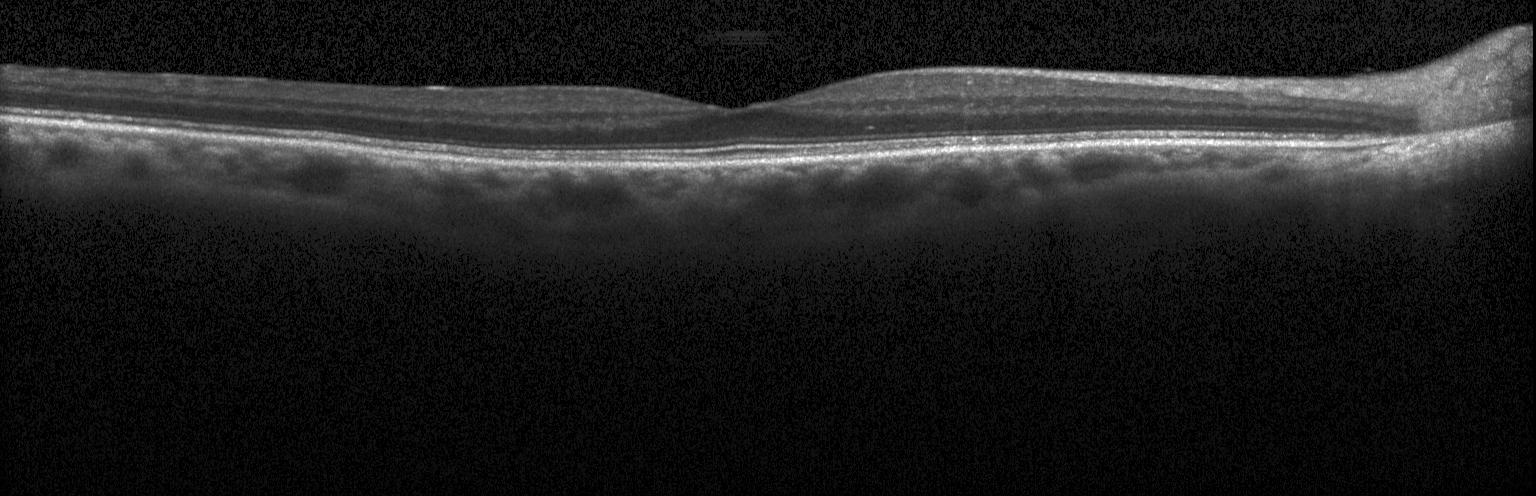
Acquired on a Heidelberg Spectralis · horizontal scan through the fovea · spectral-domain OCT · OCT B-scan
This B-scan demonstrates no choroidal neovascularization, no diabetic macular edema, and no drusen.